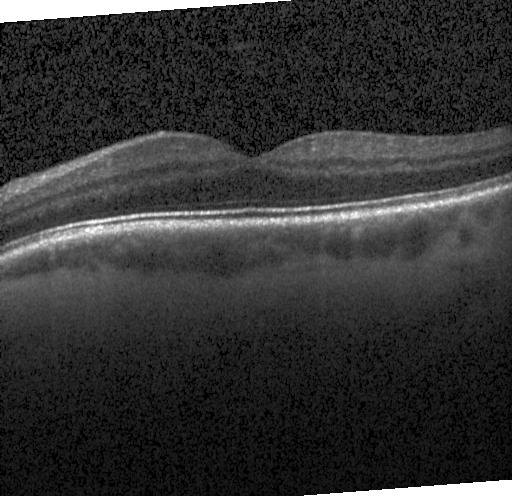 Acquired on a Heidelberg Spectralis. Fovea-centered. Spectral-domain optical coherence tomography. Retinal OCT cross-section. Finding: no evidence of CNV, DME, or drusen.